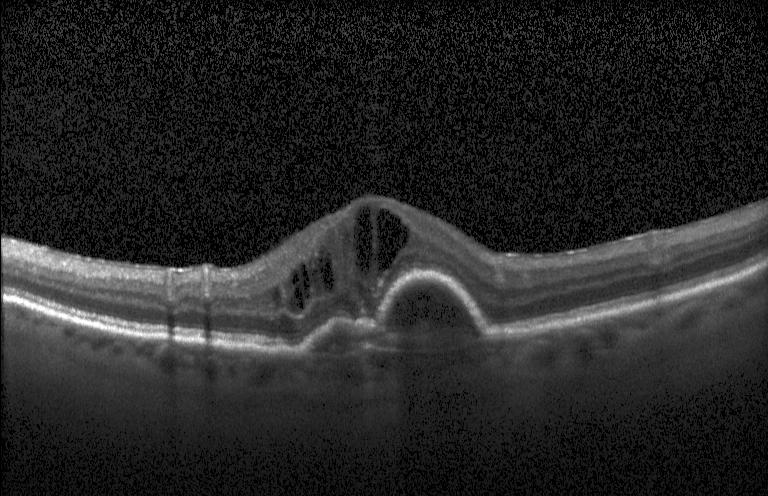

Spectral-domain optical coherence tomography, retinal OCT cross-section, instrument: Heidelberg Spectralis, fovea-centered. This B-scan demonstrates a choroidal neovascular membrane.